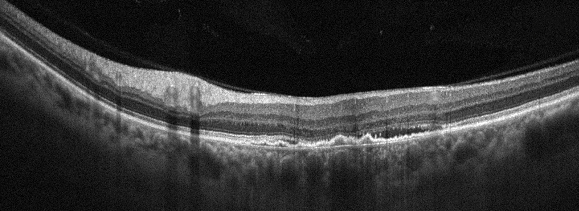

Retinal OCT cross-section, OS
This B-scan demonstrates AMD.